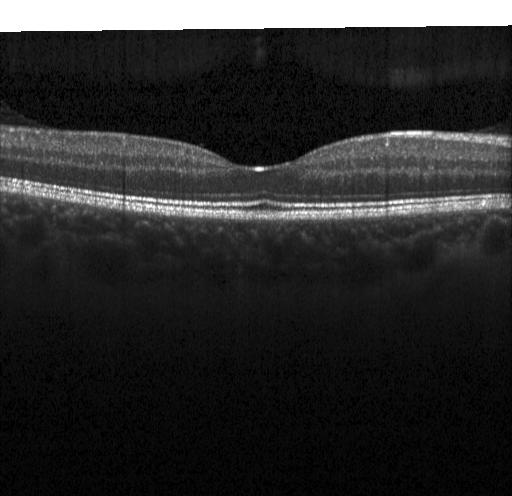 OCT B-scan.
OCT finding: no choroidal neovascularization, no diabetic macular edema, and no drusen.